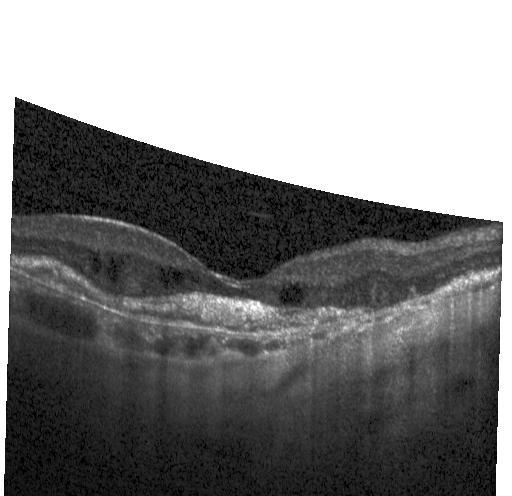
Impression: CNV.